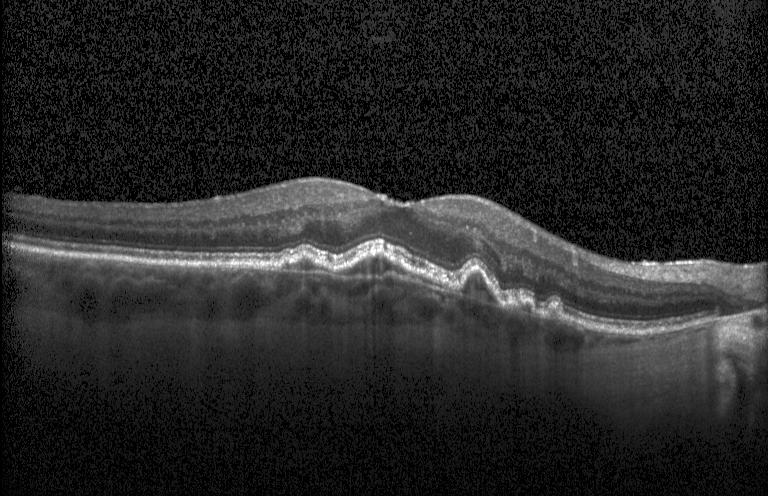 OCT B-scan; acquired on a Heidelberg Spectralis — Diagnosis: choroidal neovascularization (CNV).